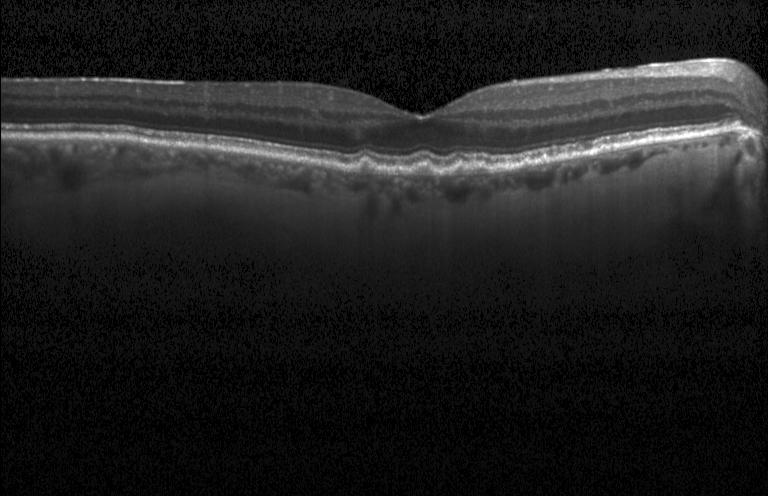
Optical coherence tomography B-scan — Macular OCT: multiple drusen.